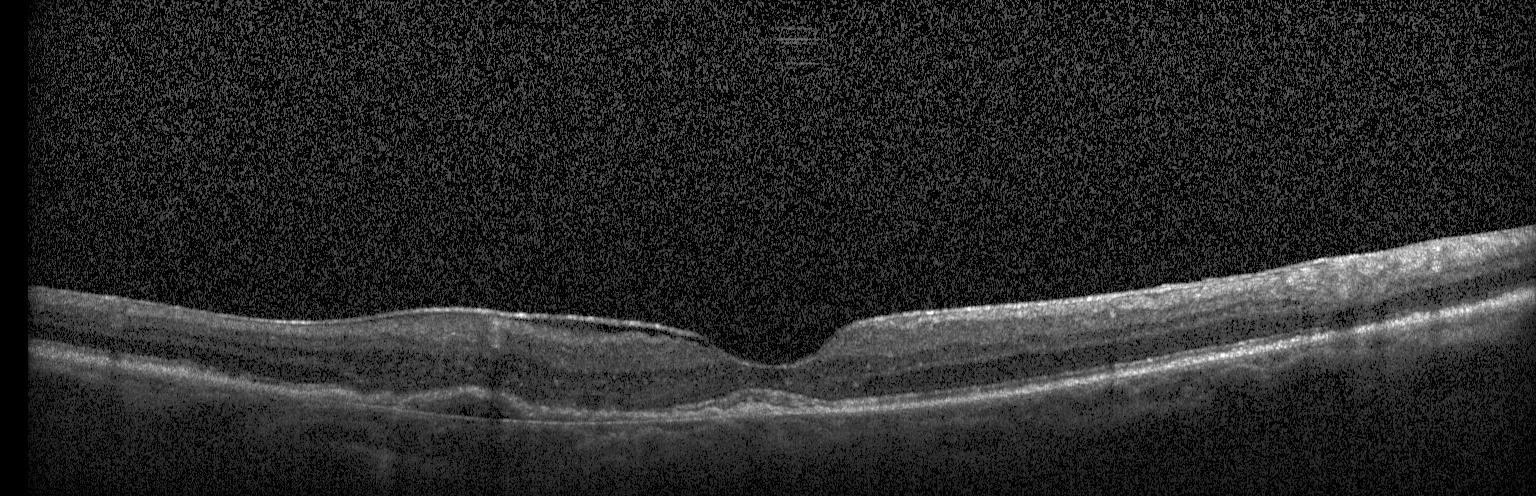 Retinal OCT B-scan; Heidelberg Spectralis — A choroidal neovascular membrane.